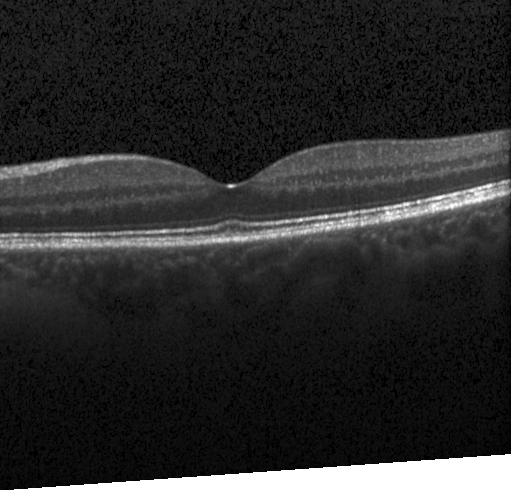
Fovea-centered · spectral-domain optical coherence tomography · retinal OCT B-scan. Finding: neither choroidal neovascularization, diabetic macular edema, nor drusen.